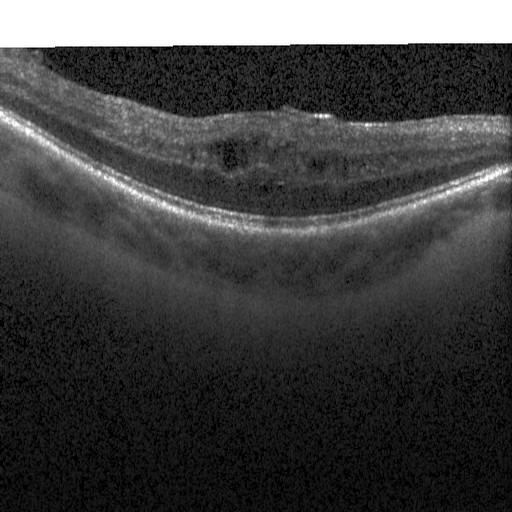
Finding: DME.